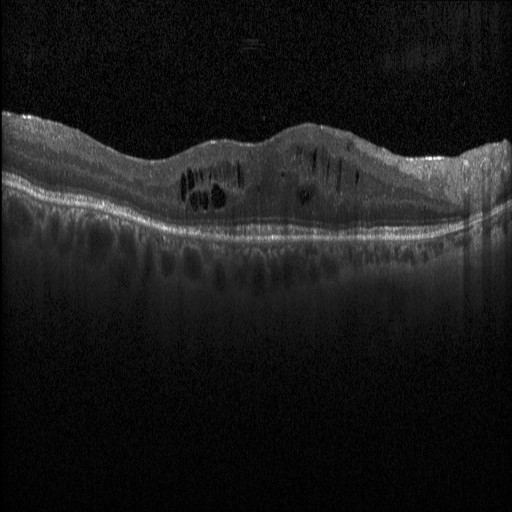

OCT finding: diabetic macular edema.